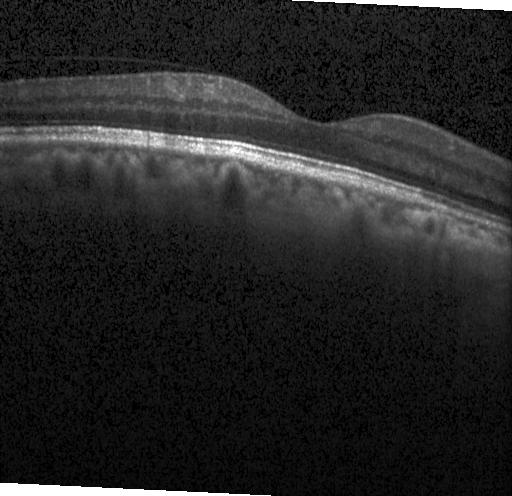 Retinal OCT cross-section · Heidelberg Spectralis · through the macula · spectral-domain OCT.
This B-scan demonstrates no CNV, no DME, and no drusen.